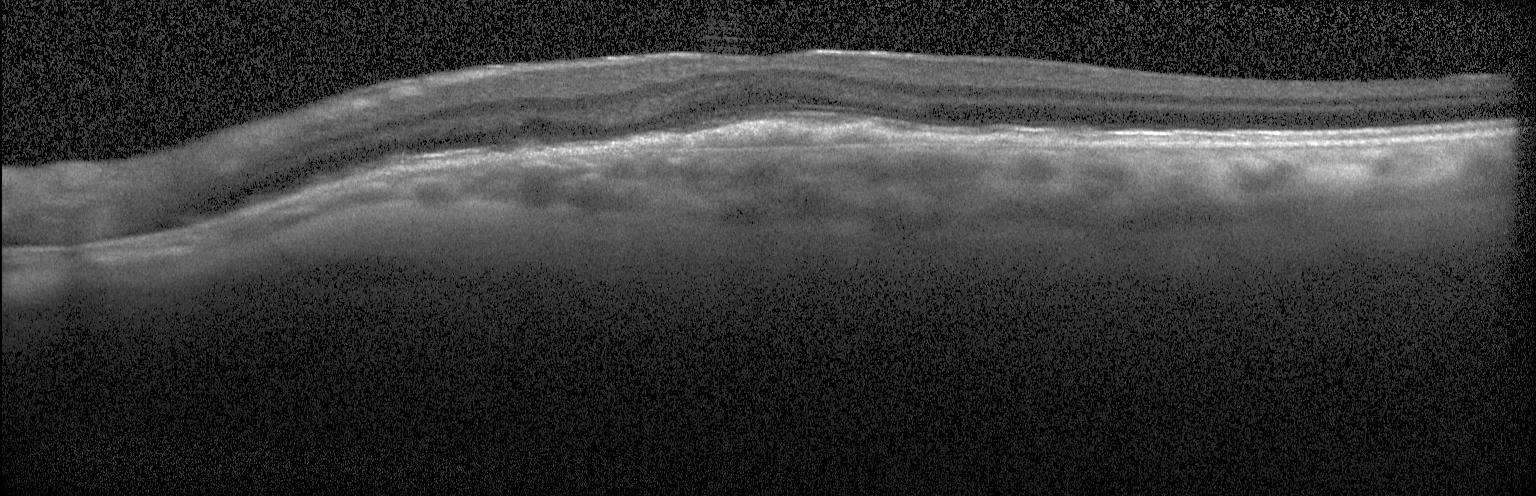

This B-scan demonstrates a choroidal neovascular membrane.